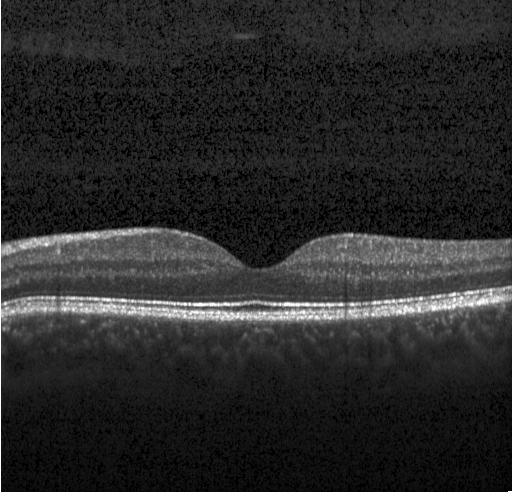

Retinal OCT B-scan. Heidelberg Spectralis. Spectral-domain OCT — Impression: no CNV, no DME, and no drusen.